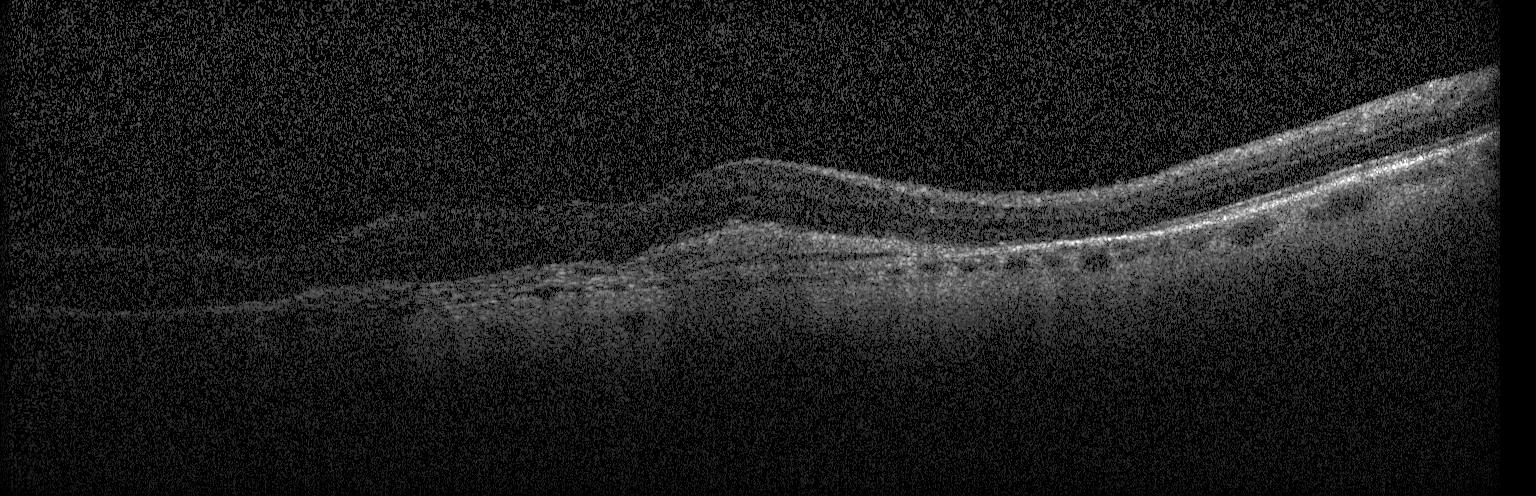 Heidelberg Spectralis OCT system · spectral-domain OCT · OCT line scan · through the macula — Choroidal neovascularization.